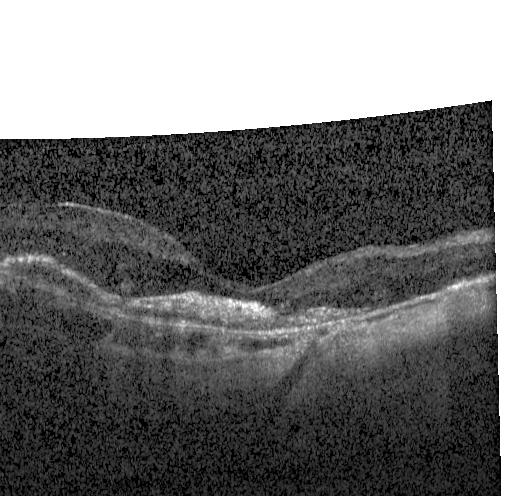
Diagnosis: choroidal neovascularization.